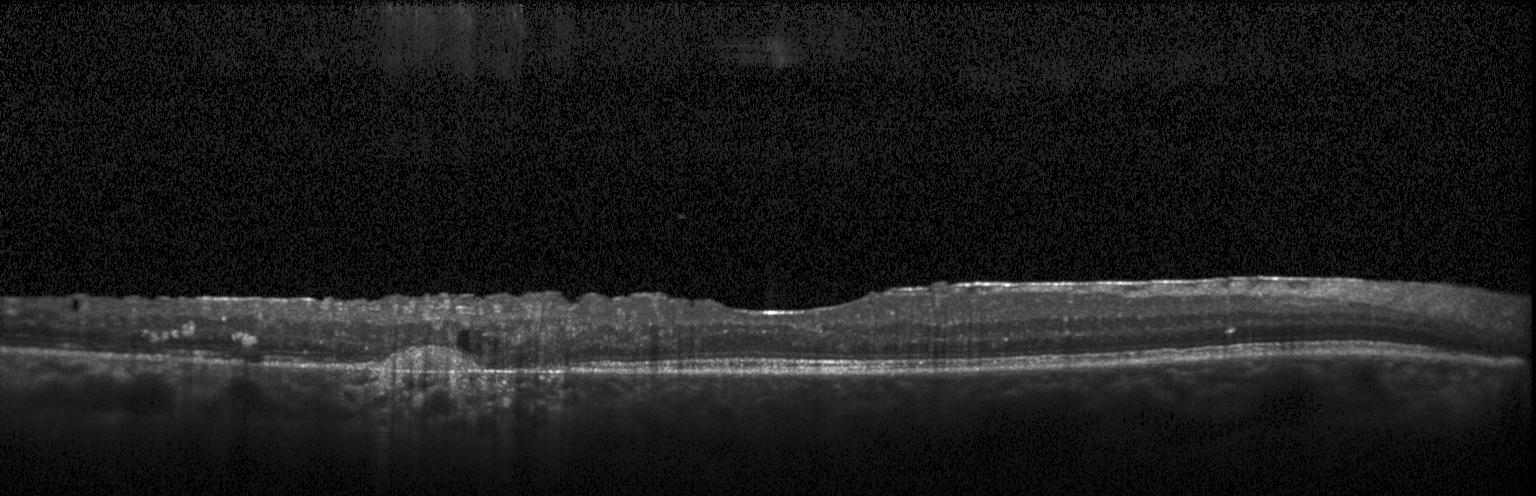 OCT line scan, through the macula, Heidelberg Spectralis. Diagnosis: a choroidal neovascular membrane.